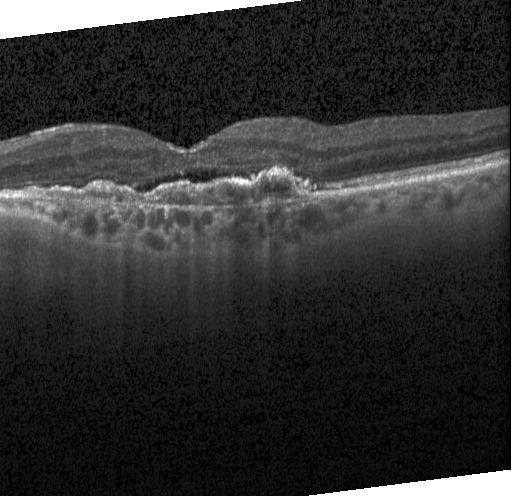

Spectral-domain OCT. Centered on the fovea. Acquired on a Heidelberg Spectralis. OCT B-scan. OCT finding: a choroidal neovascular membrane.